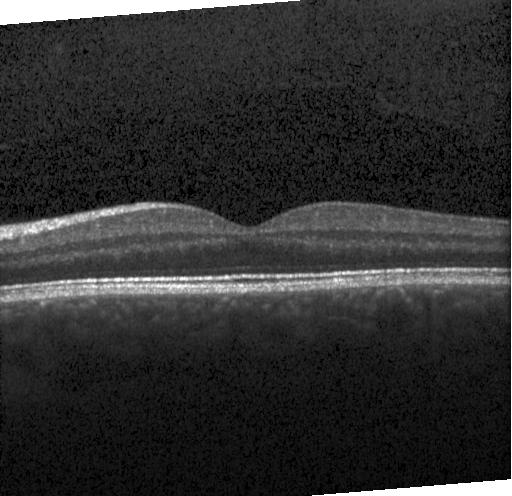
Optical coherence tomography B-scan · horizontal scan through the fovea
Impression: neither CNV, DME, nor drusen.